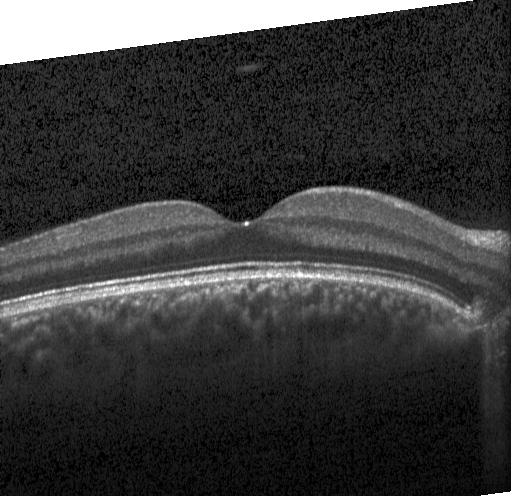 Fovea-centered · OCT B-scan — Finding: no choroidal neovascularization, no diabetic macular edema, and no drusen.